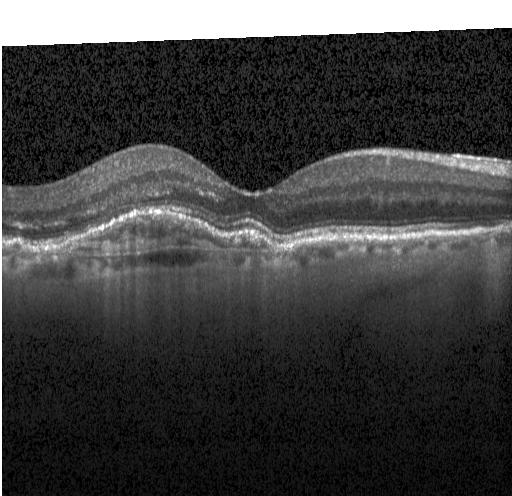
Through the macula. SD-OCT. Retinal OCT B-scan. Acquired on a Heidelberg Spectralis
Finding: a choroidal neovascular membrane.